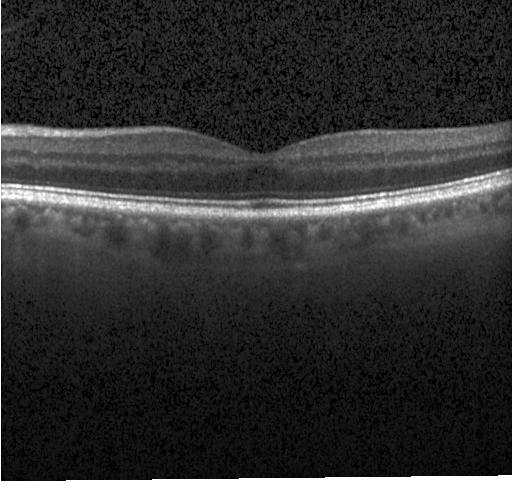

Assessment: no evidence of CNV, DME, or drusen.